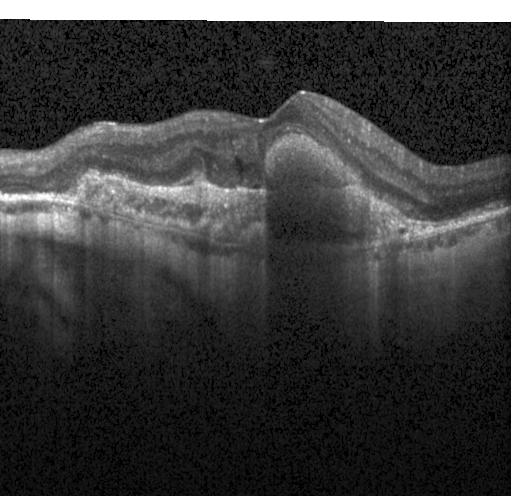

The scan shows choroidal neovascularization (CNV).